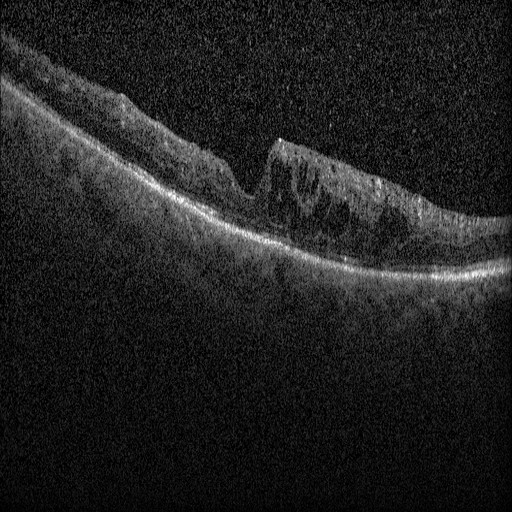

Heidelberg Spectralis; spectral-domain OCT; optical coherence tomography scan — This B-scan demonstrates diabetic macular edema.